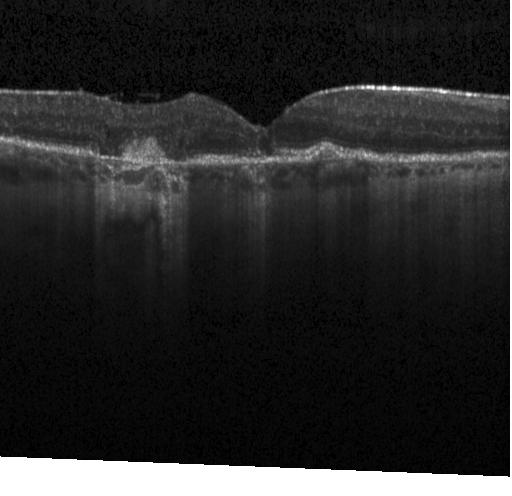
OCT B-scan showing a choroidal neovascular membrane.